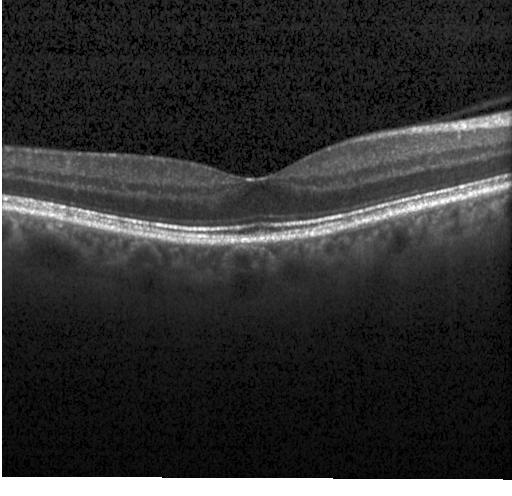

Instrument: Heidelberg Spectralis · OCT line scan · macular scan · spectral-domain optical coherence tomography — Finding: no CNV, no DME, and no drusen.